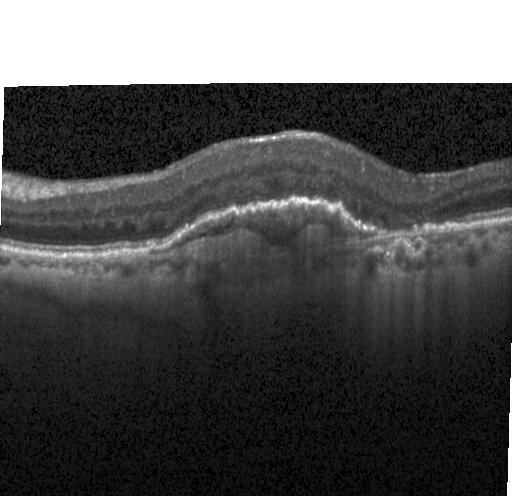 SD-OCT, fovea-centered, OCT B-scan, Heidelberg Spectralis — The scan shows choroidal neovascularization.